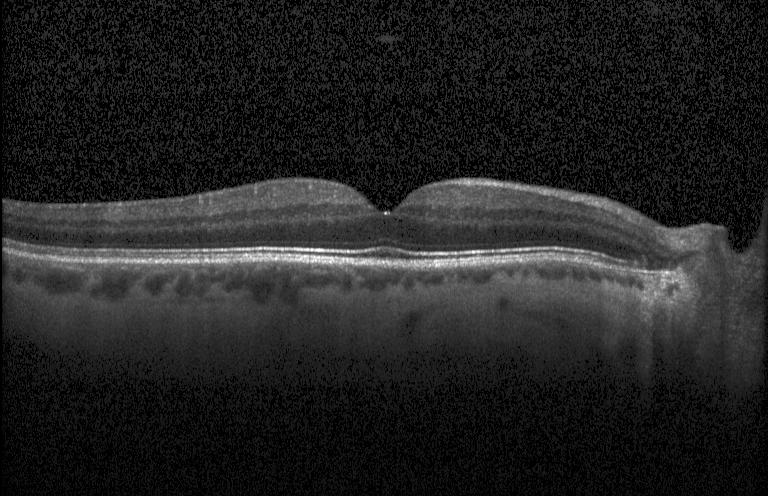 Impression: neither CNV, DME, nor drusen.